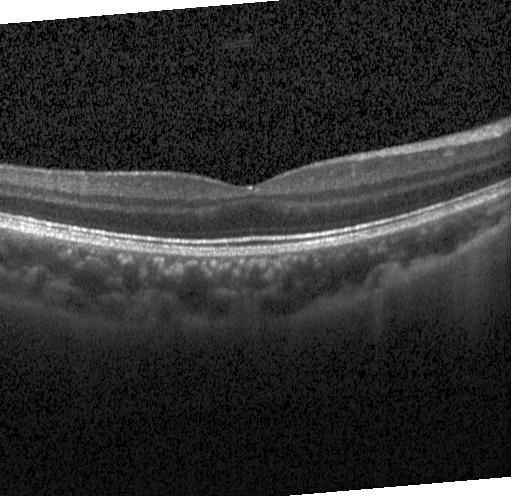
Macular scan; spectral-domain OCT; acquired on a Heidelberg Spectralis; optical coherence tomography B-scan.
The scan shows neither choroidal neovascularization, diabetic macular edema, nor drusen.